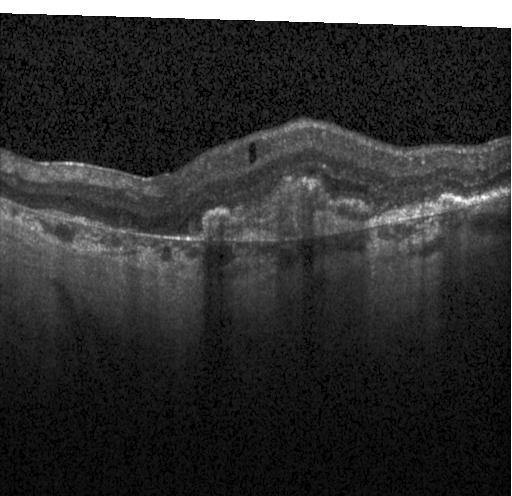
Spectral-domain optical coherence tomography; optical coherence tomography B-scan; fovea-centered. The scan shows a choroidal neovascular membrane.